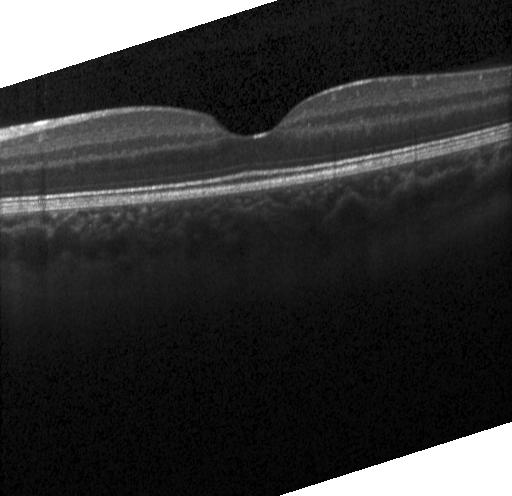 Macular scan. Spectral-domain optical coherence tomography. Heidelberg Spectralis OCT system. Optical coherence tomography scan
Neither CNV, DME, nor drusen.